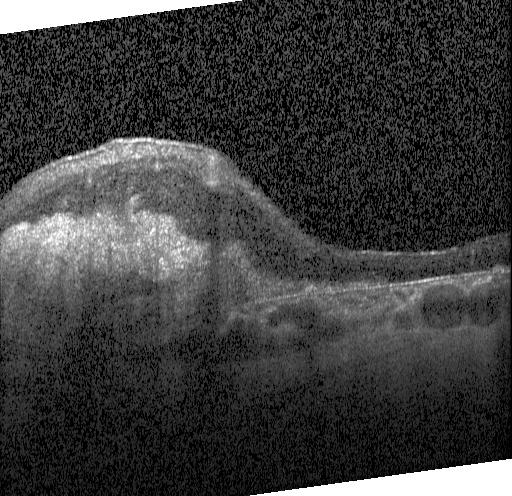
Choroidal neovascularization.